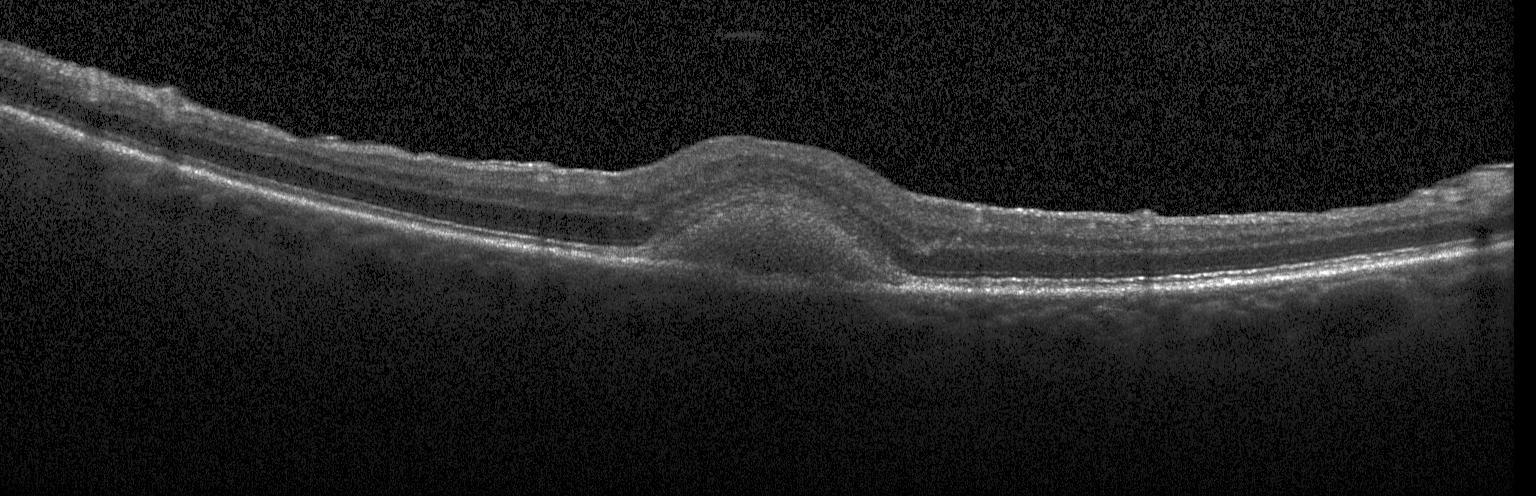

Impression: a choroidal neovascular membrane.